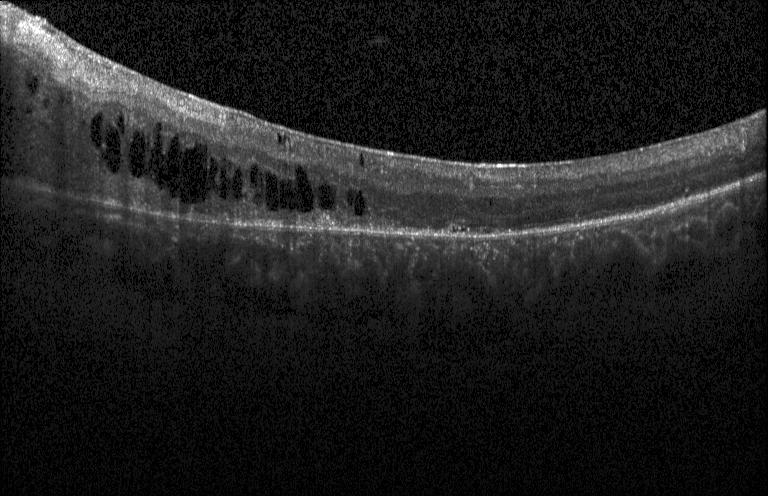
SD-OCT; Heidelberg Spectralis; optical coherence tomography B-scan; horizontal scan through the fovea
OCT finding: diabetic macular edema (DME).